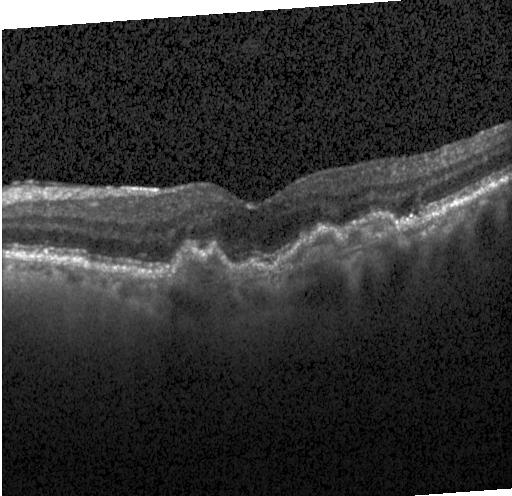 OCT B-scan; Heidelberg Spectralis; spectral-domain OCT; centered on the fovea — Dx: CNV.